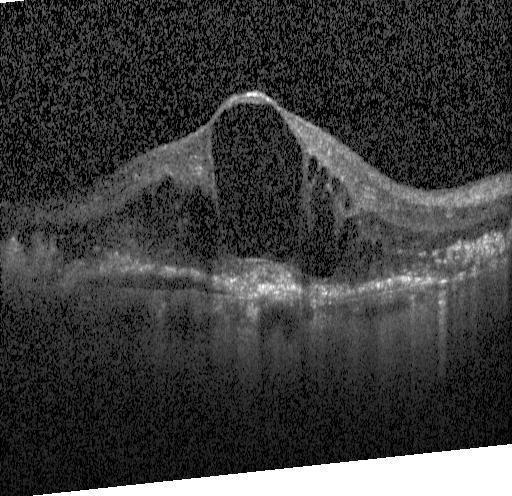

Retinal OCT cross-section. SD-OCT. Finding: a choroidal neovascular membrane.